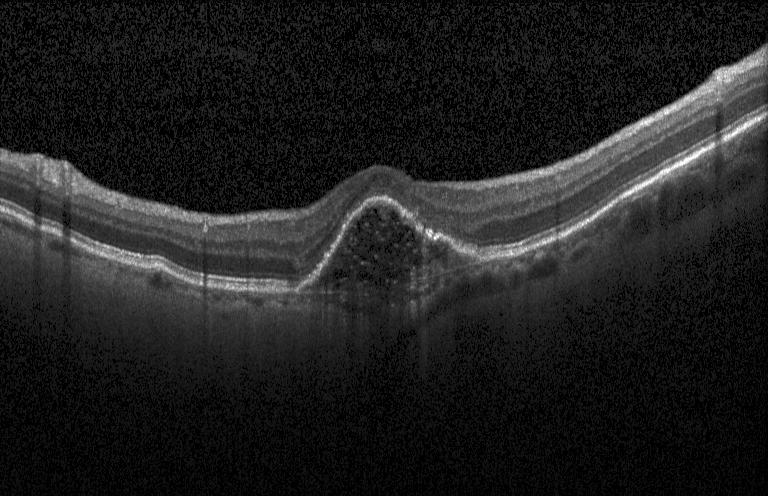 Retinal OCT B-scan. Spectral-domain OCT. The scan shows CNV.